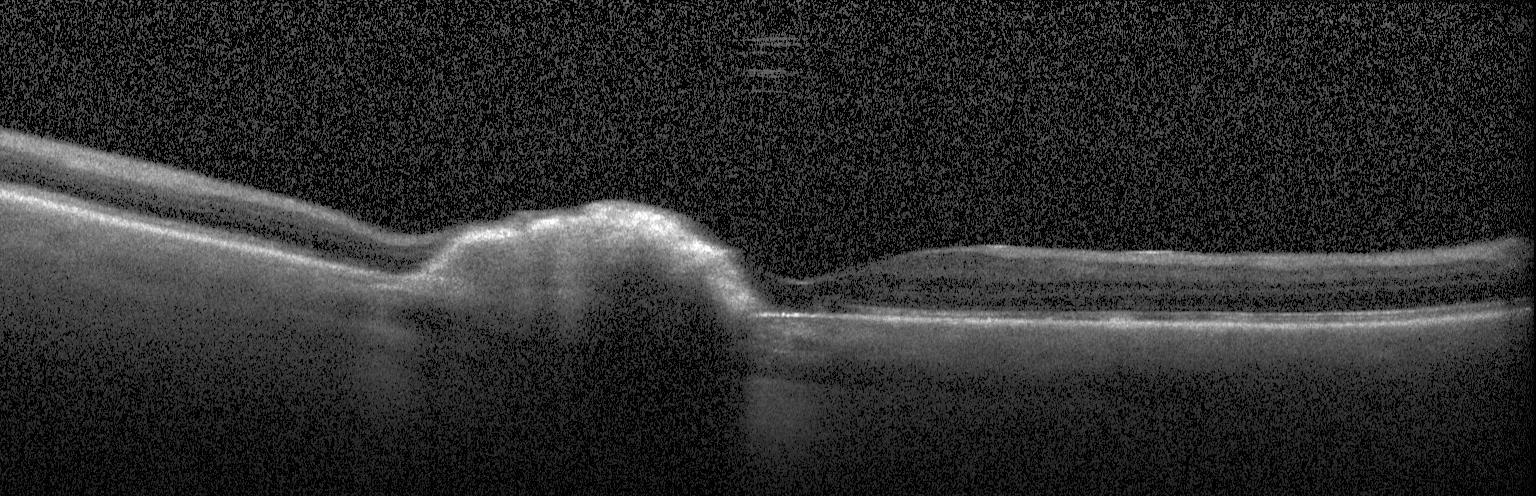 Macular scan · retinal OCT cross-section
Finding: choroidal neovascularization (CNV).